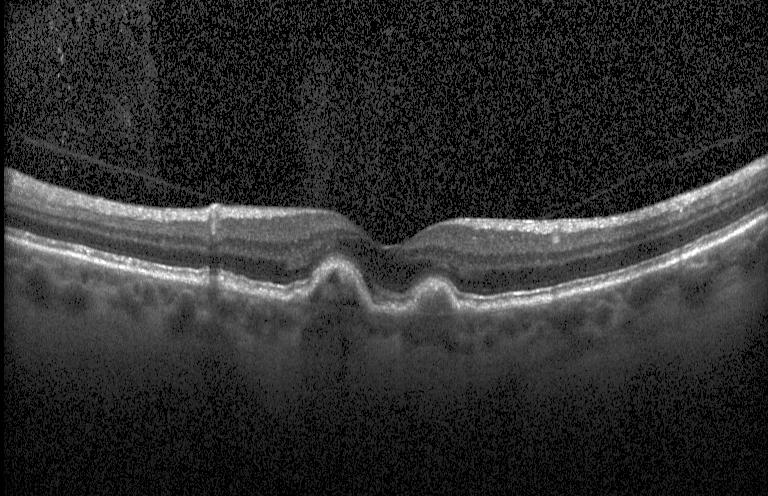 Finding: multiple drusen.